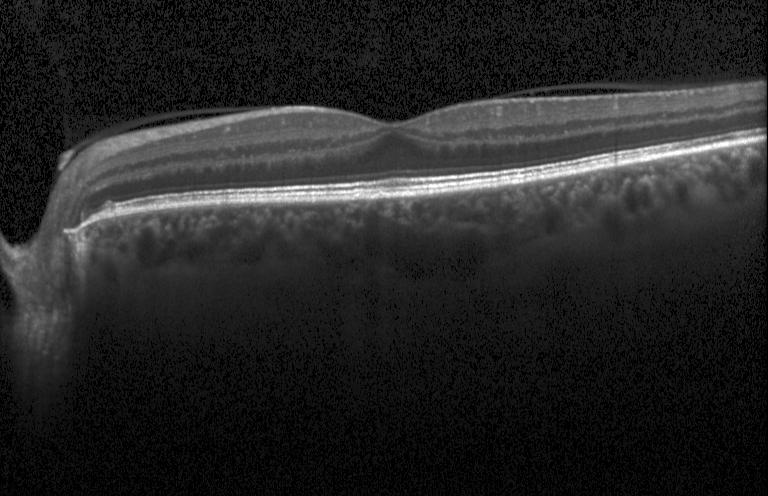 No evidence of choroidal neovascularization, diabetic macular edema, or drusen.